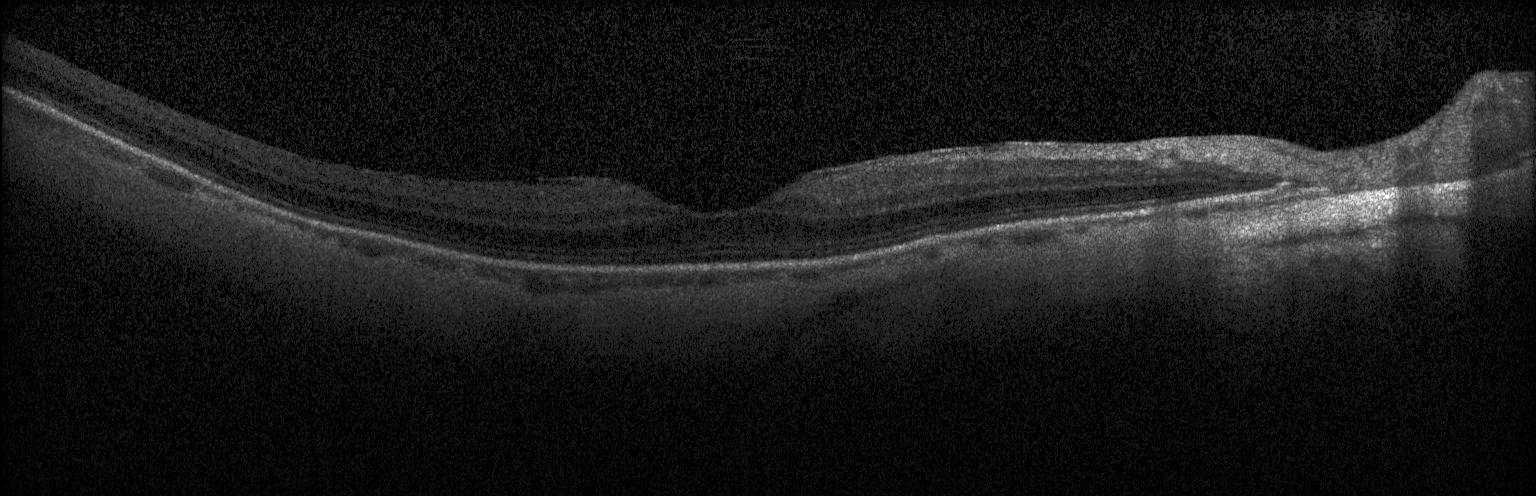 OCT finding: no evidence of choroidal neovascularization, diabetic macular edema, or drusen.